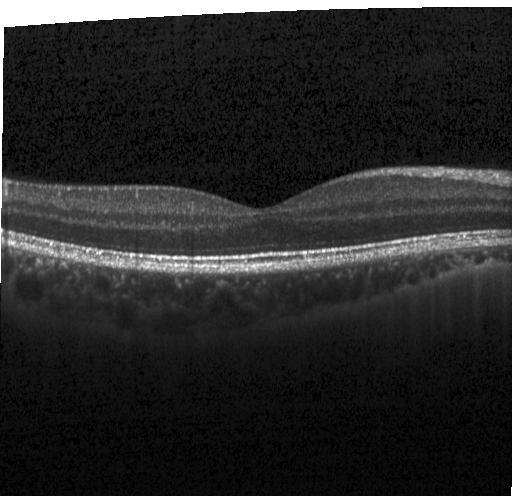 Assessment: no CNV, DME, or drusen.